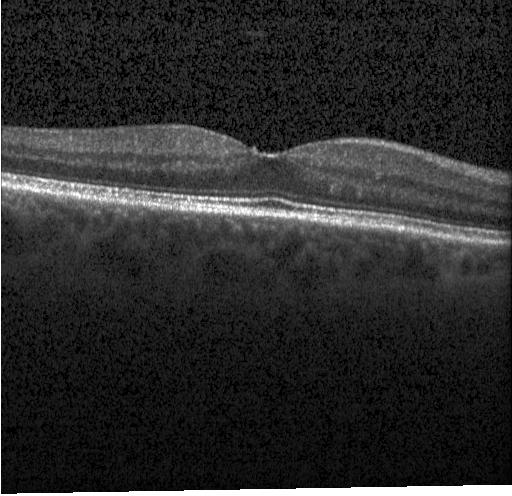

Finding: no evidence of CNV, DME, or drusen.